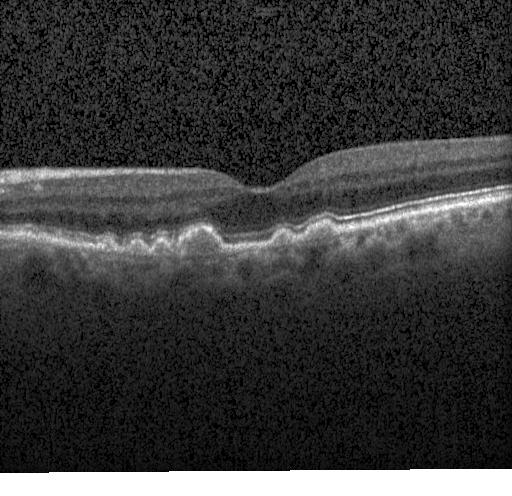

Spectral-domain OCT. Through the macula. Heidelberg Spectralis. OCT line scan. The scan shows multiple drusen.